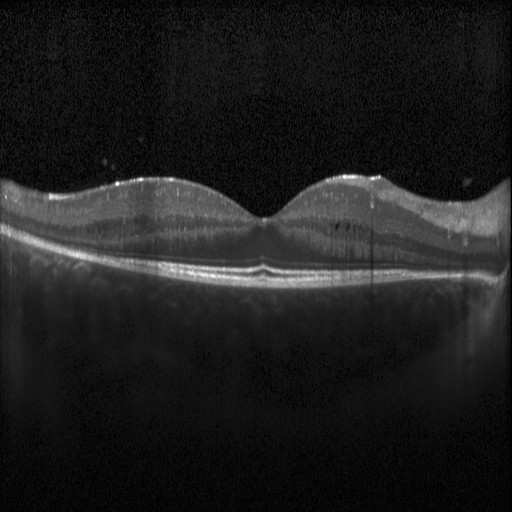 Spectral-domain OCT B-scan: DME.